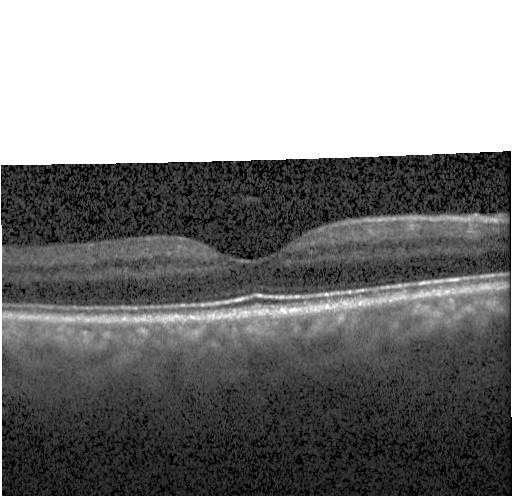

OCT scan showing neither choroidal neovascularization, diabetic macular edema, nor drusen.